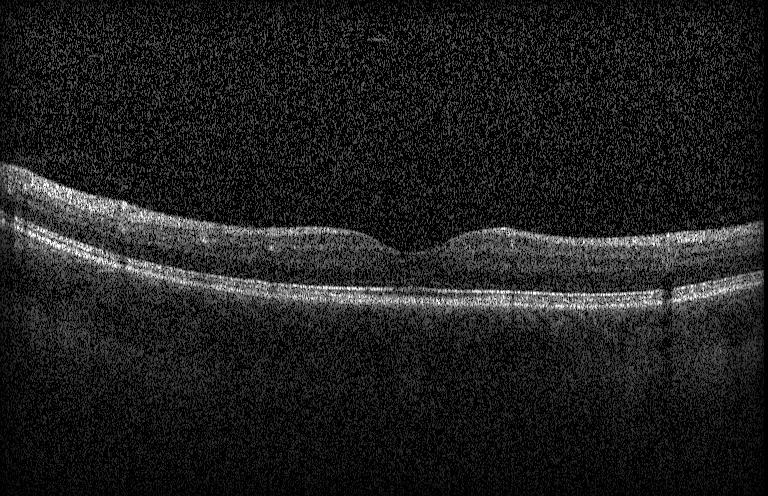
Horizontal scan through the fovea. Retinal OCT cross-section
The scan shows neither choroidal neovascularization, diabetic macular edema, nor drusen.